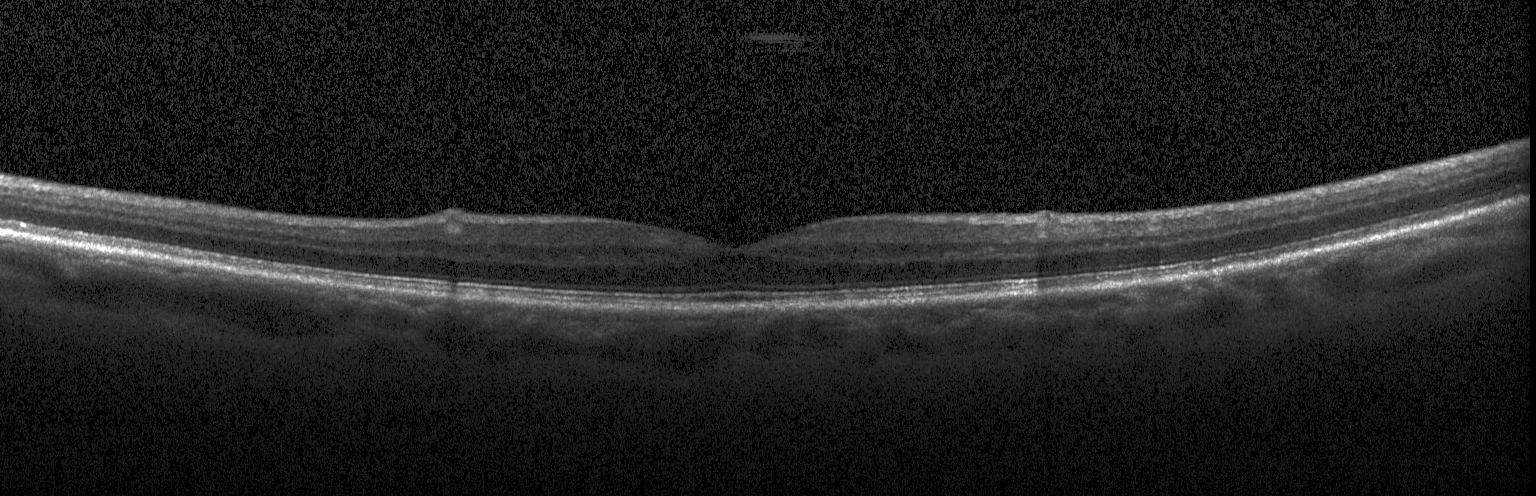

Horizontal scan through the fovea, retinal OCT cross-section.
Diagnosis: no evidence of choroidal neovascularization, diabetic macular edema, or drusen.